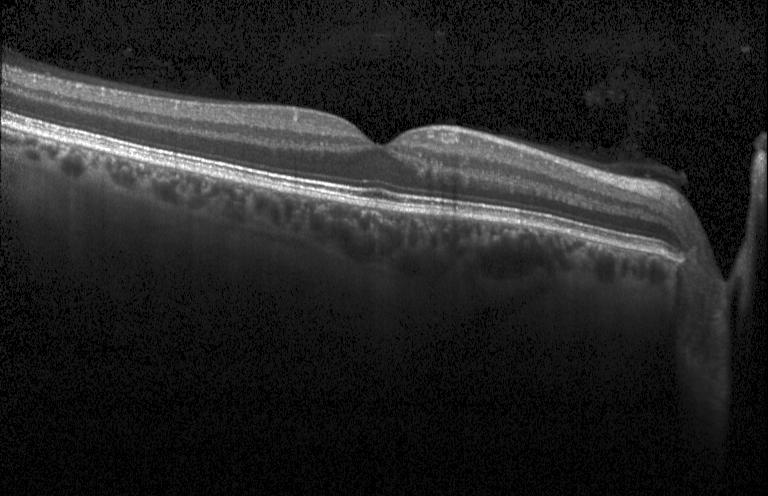 Retinal OCT B-scan — Impression: neither choroidal neovascularization, diabetic macular edema, nor drusen.